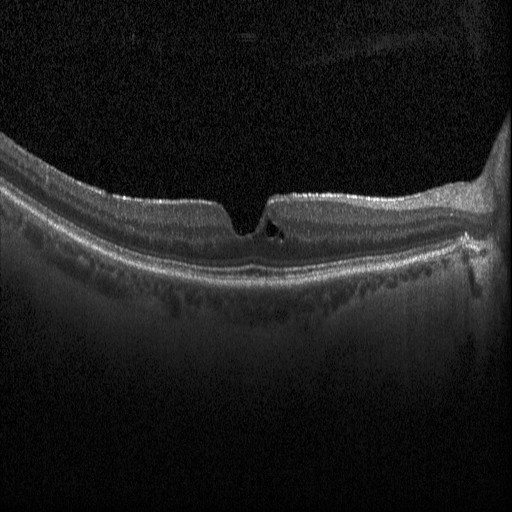 Finding: diabetic macular edema.